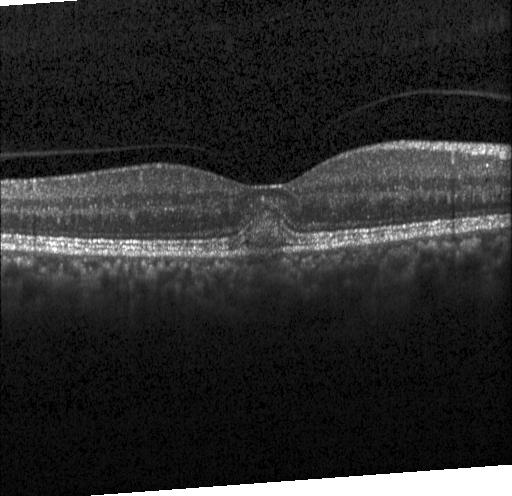

OCT scan showing a choroidal neovascular membrane.